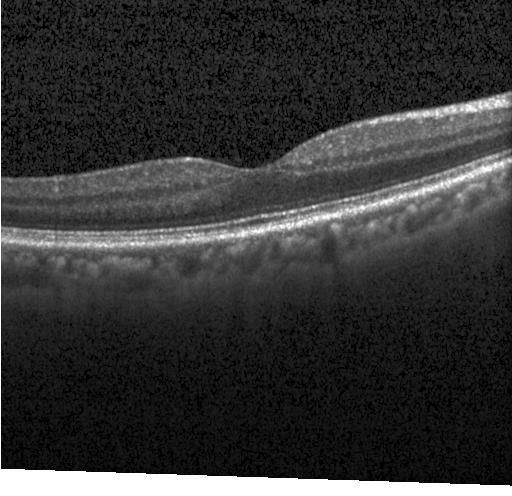
Horizontal scan through the fovea, acquired on a Heidelberg Spectralis, retinal OCT B-scan.
The scan shows no evidence of choroidal neovascularization, diabetic macular edema, or drusen.